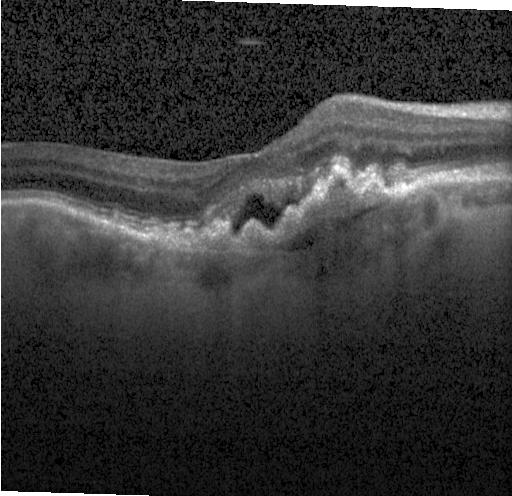
Fovea-centered · OCT line scan — Impression: CNV.